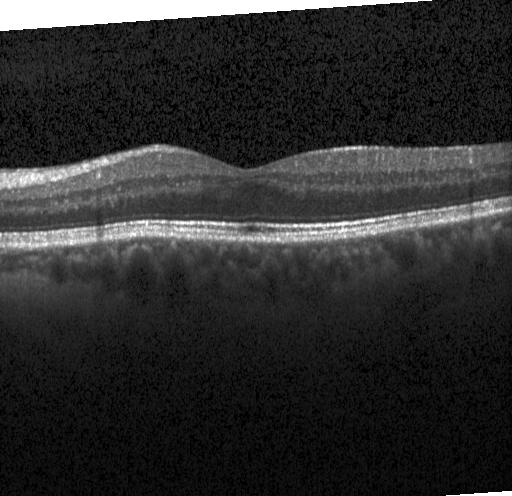
OCT B-scan showing no choroidal neovascularization, diabetic macular edema, or drusen.